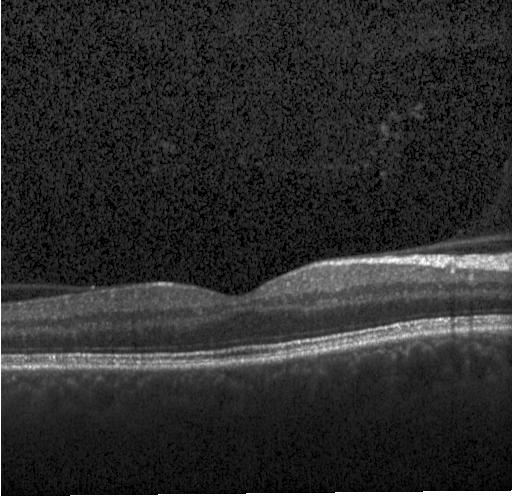 This B-scan demonstrates no choroidal neovascularization, diabetic macular edema, or drusen.